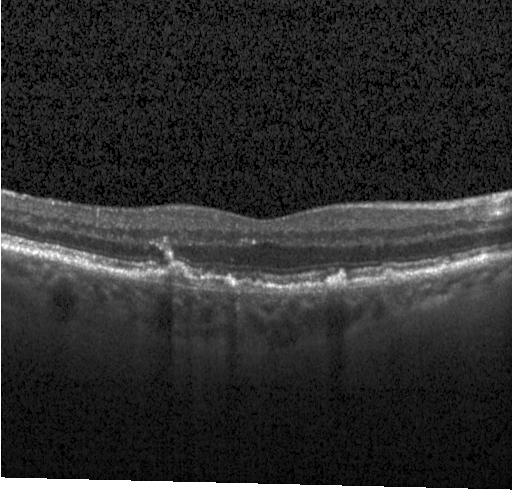

Spectral-domain OCT B-scan: a choroidal neovascular membrane.